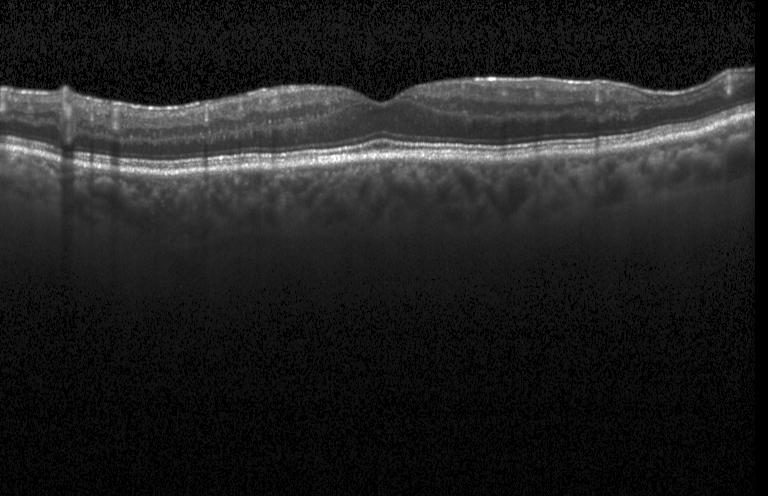 OCT line scan.
Assessment: no evidence of choroidal neovascularization, diabetic macular edema, or drusen.